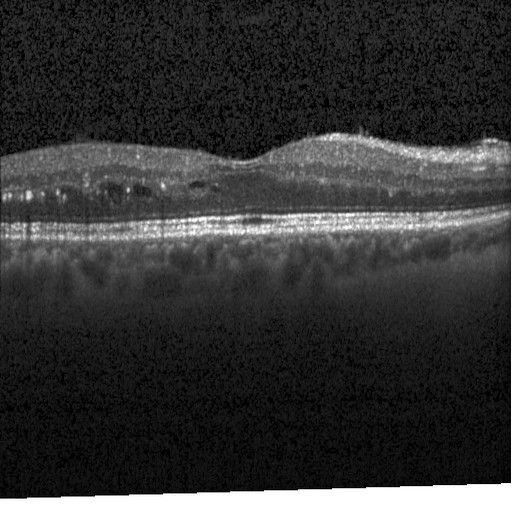

Impression: DME.